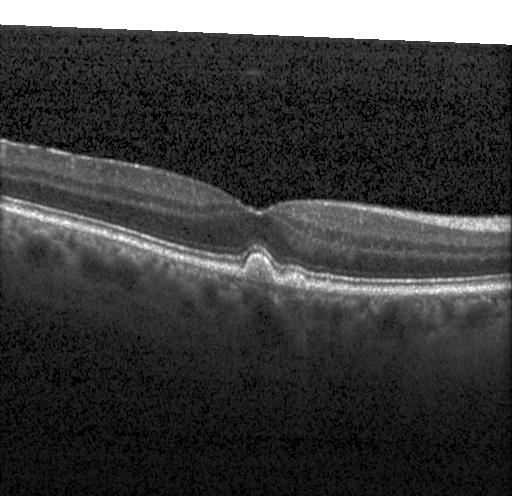

The scan shows sub-RPE drusenoid deposits.